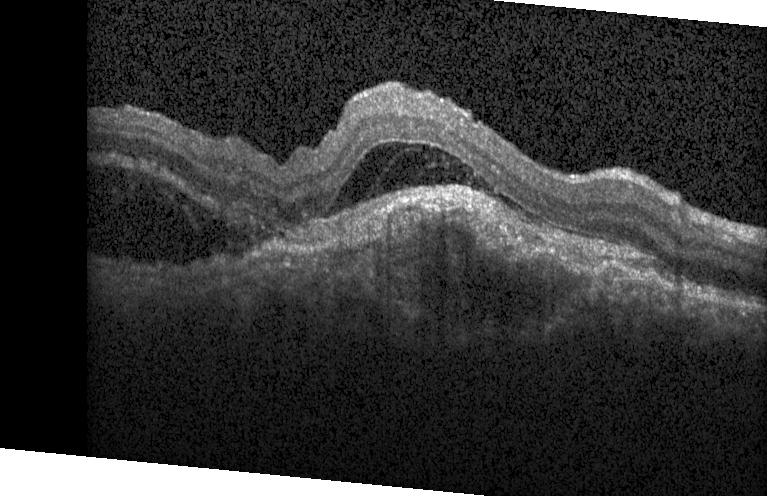 Dx: a choroidal neovascular membrane.